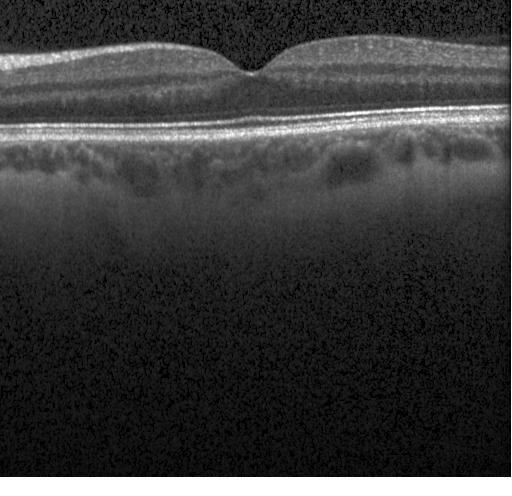 Impression: neither choroidal neovascularization, diabetic macular edema, nor drusen.